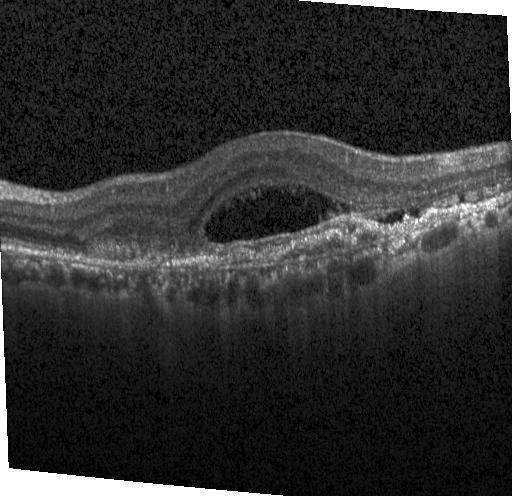 This B-scan demonstrates choroidal neovascularization (CNV).